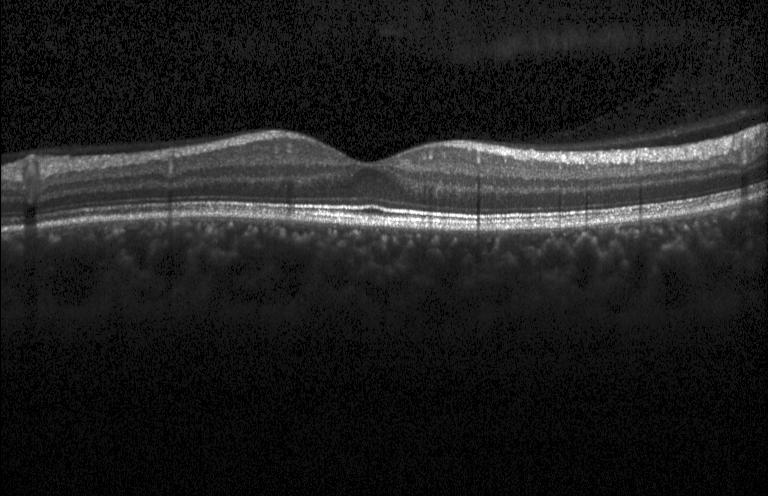 Heidelberg Spectralis OCT system · fovea-centered · optical coherence tomography B-scan. Impression: no choroidal neovascularization, no diabetic macular edema, and no drusen.